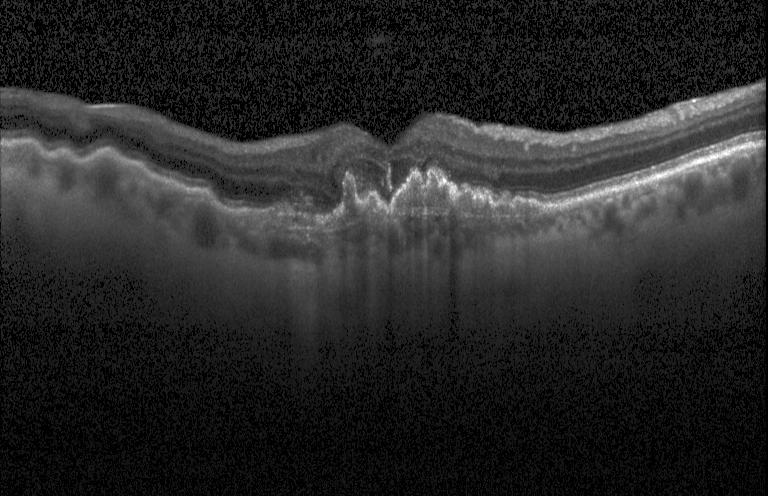

Finding: a choroidal neovascular membrane.